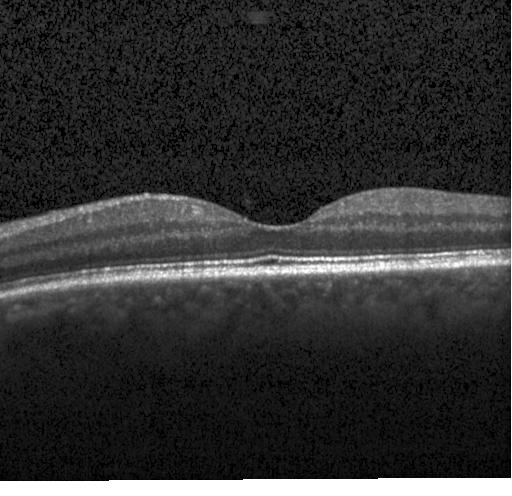

OCT B-scan — Neither choroidal neovascularization, diabetic macular edema, nor drusen.